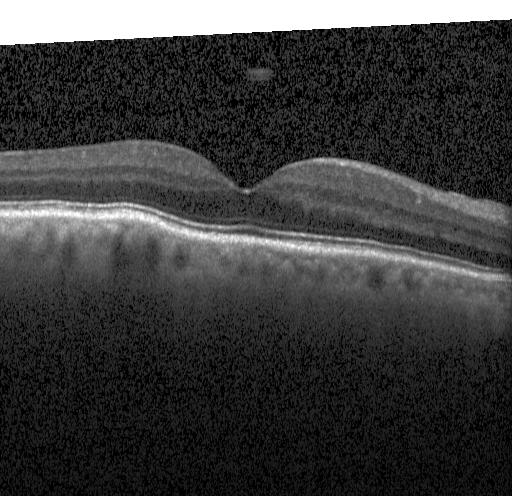
Macular OCT demonstrating no choroidal neovascularization, no diabetic macular edema, and no drusen.